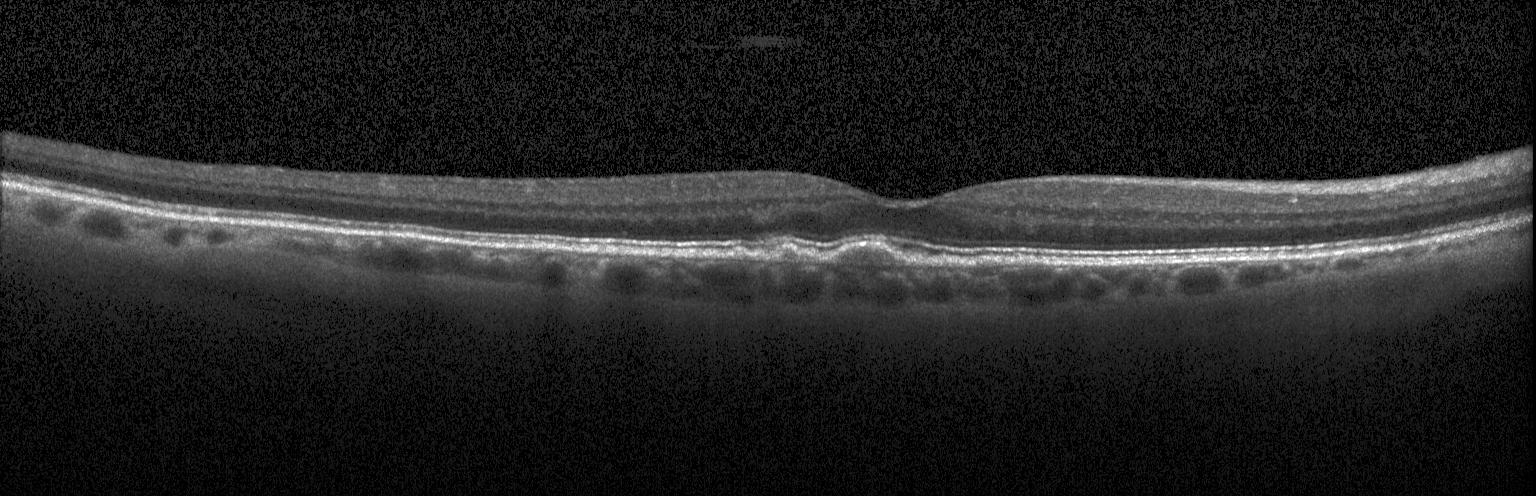

Spectral-domain optical coherence tomography; retinal OCT B-scan.
Assessment: multiple drusen.